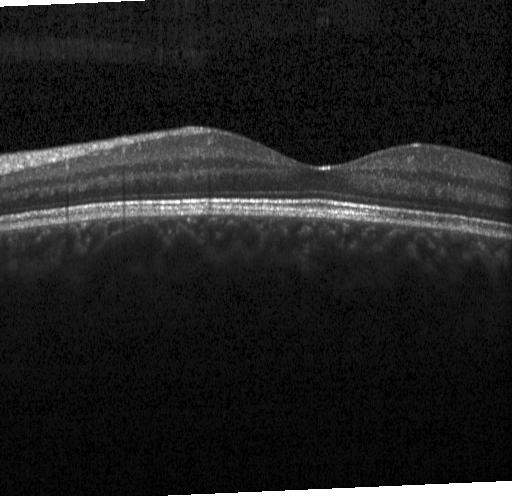
Retinal OCT cross-section · SD-OCT · horizontal scan through the fovea · acquired on a Heidelberg Spectralis. Dx: no evidence of choroidal neovascularization, diabetic macular edema, or drusen.